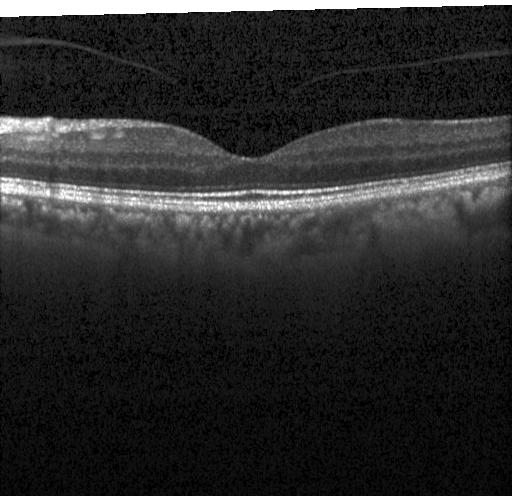

Spectral-domain optical coherence tomography; retinal OCT cross-section; Heidelberg Spectralis OCT system. Diagnosis: neither CNV, DME, nor drusen.